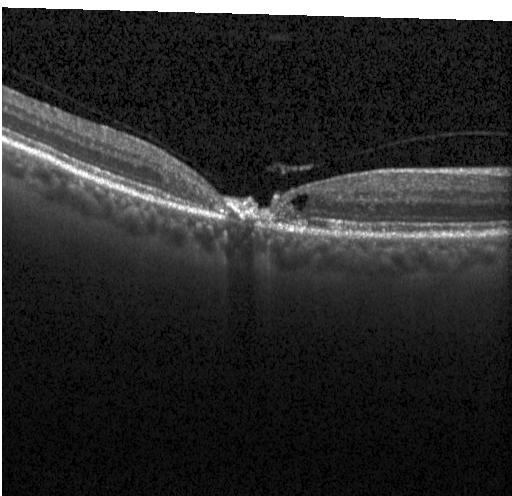
Impression: CNV.